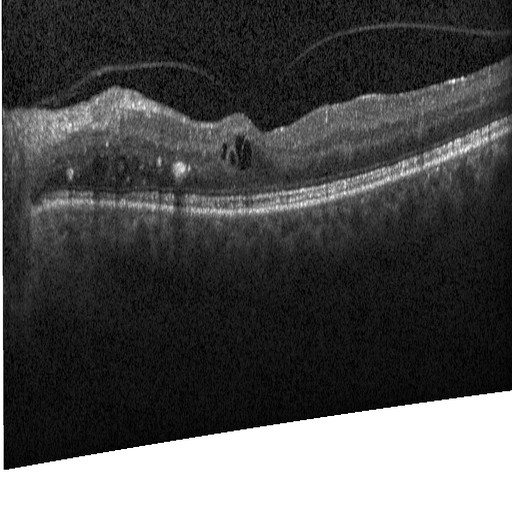 Centered on the fovea. Optical coherence tomography scan.
Dx: diabetic macular edema.